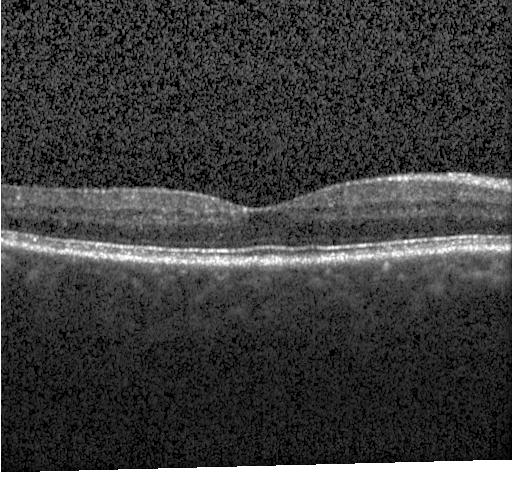 Through the macula; acquired on a Heidelberg Spectralis; optical coherence tomography scan — The scan shows neither choroidal neovascularization, diabetic macular edema, nor drusen.